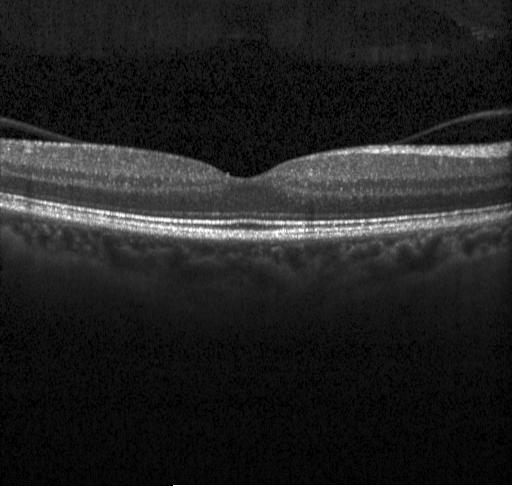

Spectral-domain OCT, retinal OCT cross-section — No evidence of choroidal neovascularization, diabetic macular edema, or drusen.